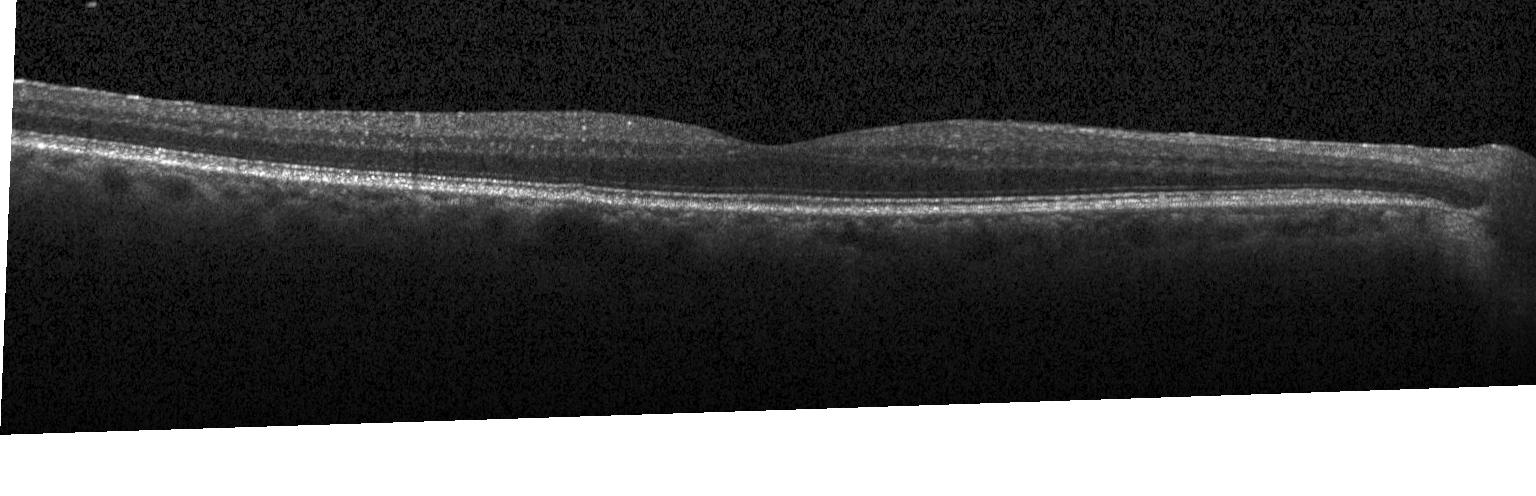

Optical coherence tomography B-scan
The scan shows no choroidal neovascularization, diabetic macular edema, or drusen.